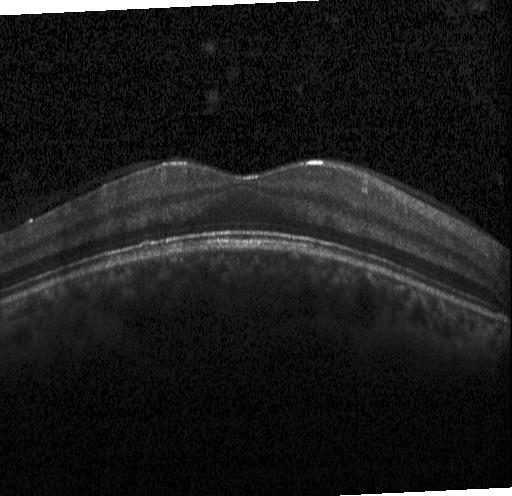

Retinal OCT cross-section · fovea-centered · acquired on a Heidelberg Spectralis · SD-OCT.
Diagnosis: no choroidal neovascularization, diabetic macular edema, or drusen.